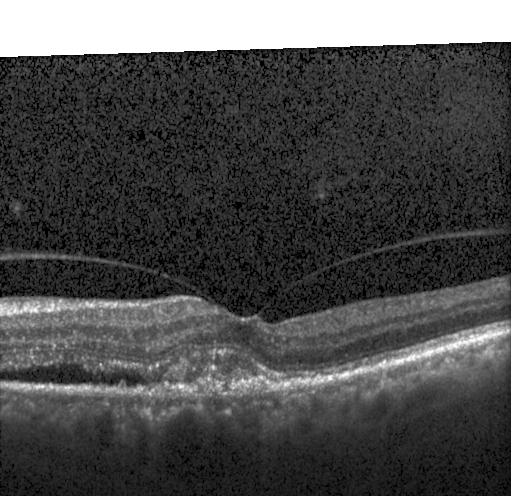

Impression: a choroidal neovascular membrane.